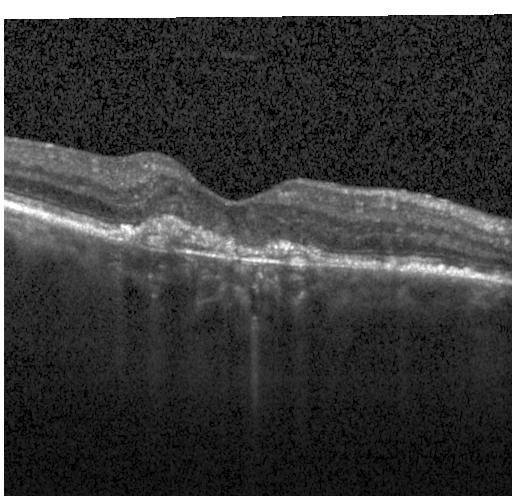
Macular OCT: CNV.